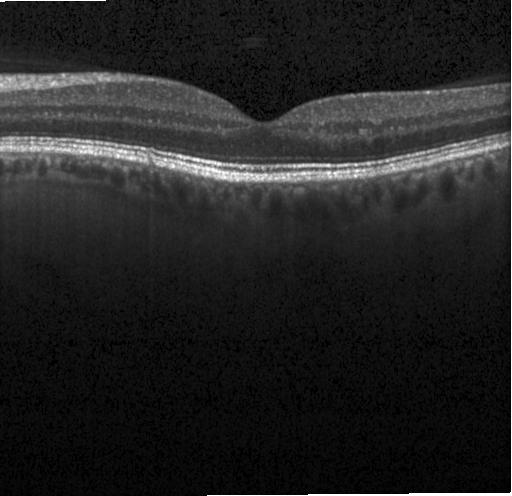
Optical coherence tomography B-scan. Diagnosis: no choroidal neovascularization, diabetic macular edema, or drusen.